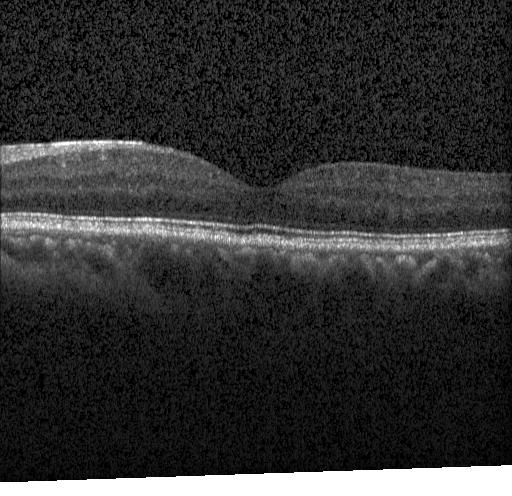 Spectral-domain OCT; acquired on a Heidelberg Spectralis; retinal OCT cross-section — The scan shows no evidence of CNV, DME, or drusen.